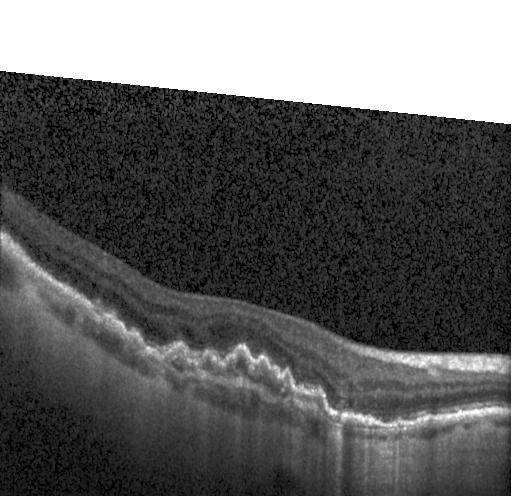

Optical coherence tomography B-scan; spectral-domain optical coherence tomography; instrument: Heidelberg Spectralis — Assessment: CNV.